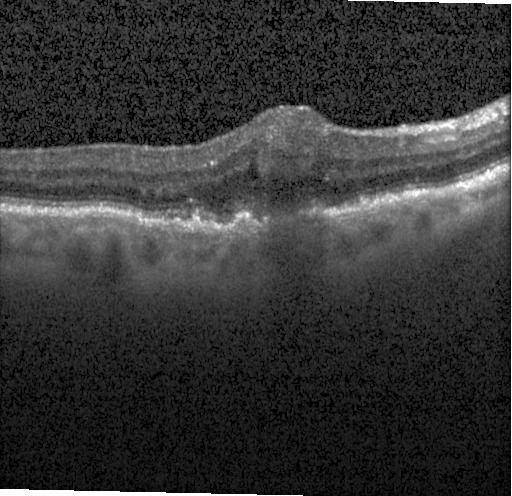
Acquired on a Heidelberg Spectralis. Optical coherence tomography scan. Horizontal scan through the fovea.
Diagnosis: CNV.